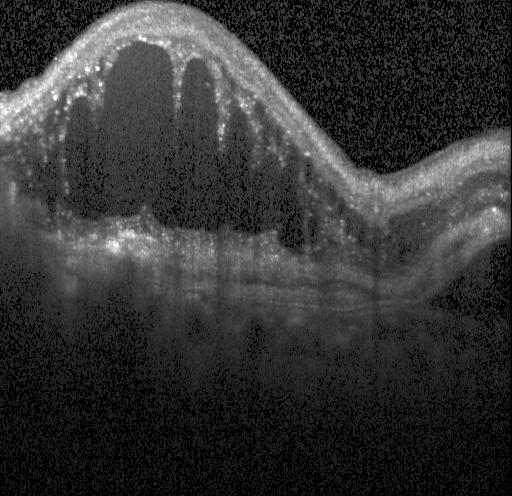

Retinal OCT B-scan — Finding: DME.